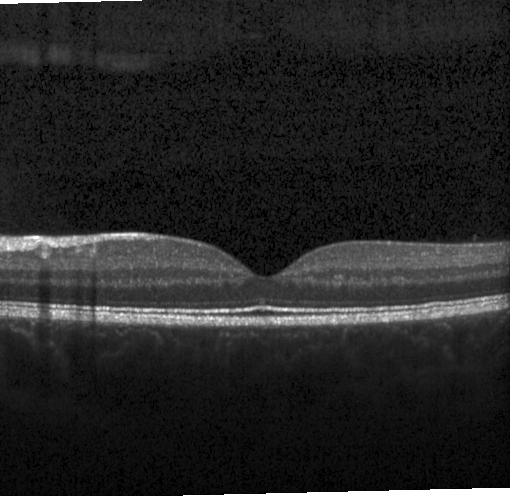

Spectral-domain optical coherence tomography; OCT line scan; Heidelberg Spectralis — No CNV, no DME, and no drusen.